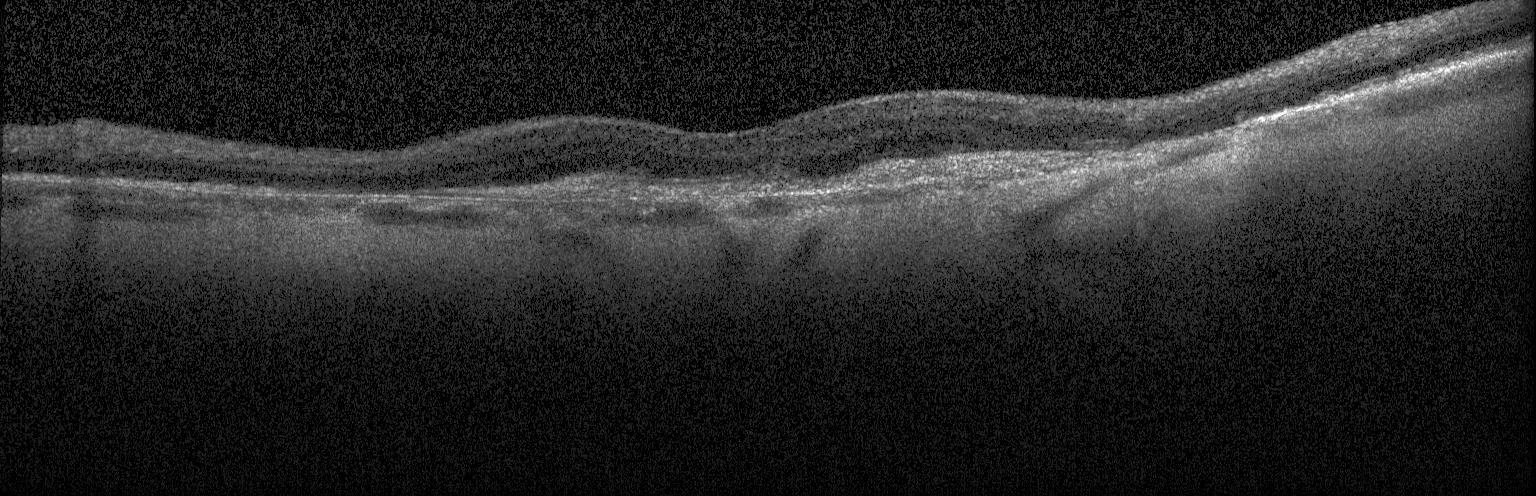

A choroidal neovascular membrane.